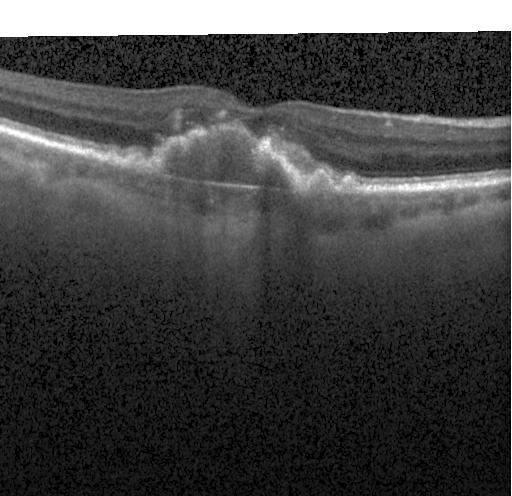

Retinal OCT cross-section.
Impression: choroidal neovascularization (CNV).